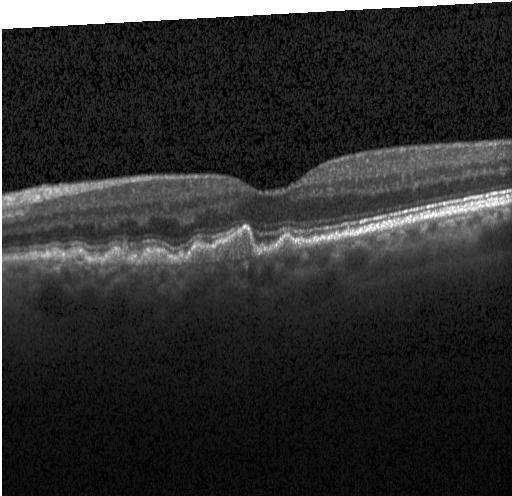

Impression: drusen.